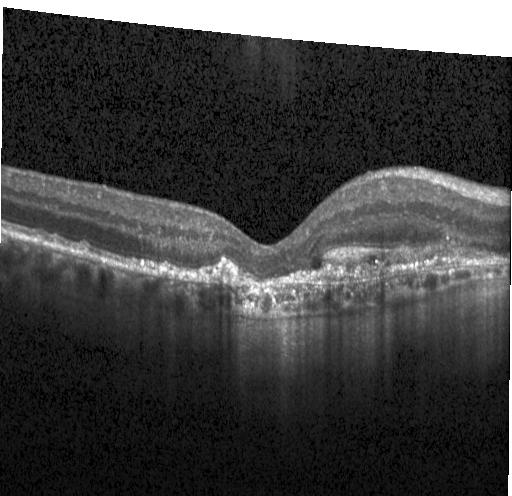 Retinal OCT cross-section
Finding: CNV.